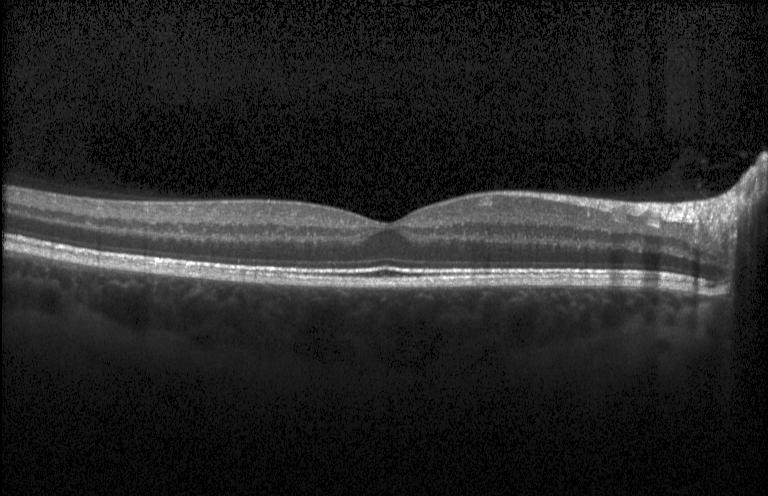

Fovea-centered; retinal OCT B-scan — Macular OCT: neither choroidal neovascularization, diabetic macular edema, nor drusen.